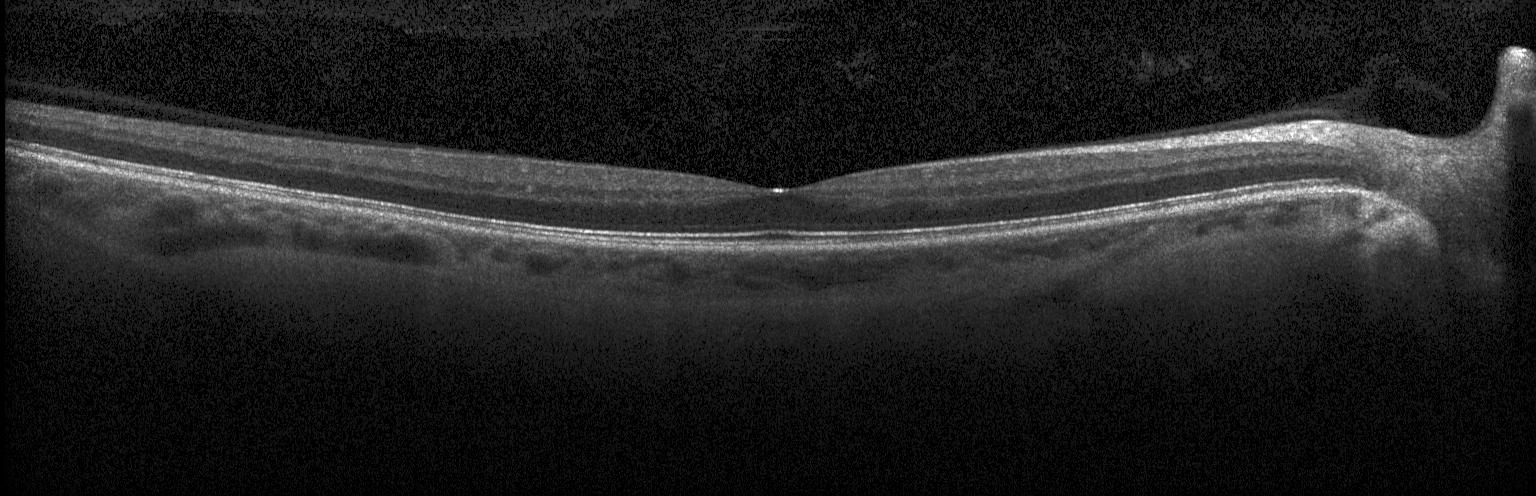
Spectral-domain OCT B-scan: no choroidal neovascularization, no diabetic macular edema, and no drusen.